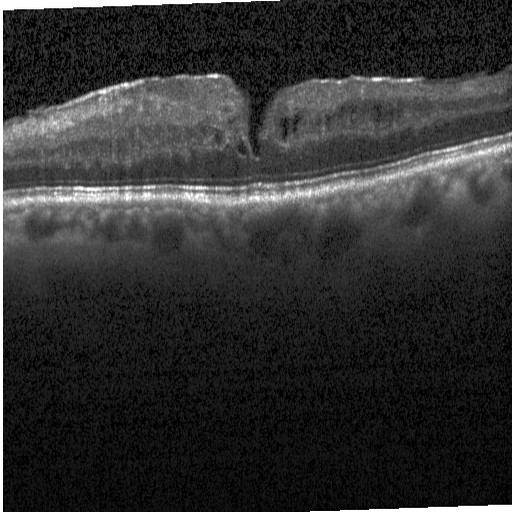 Centered on the fovea. Acquired on a Heidelberg Spectralis. Retinal OCT B-scan
Diagnosis: diabetic macular edema (DME).